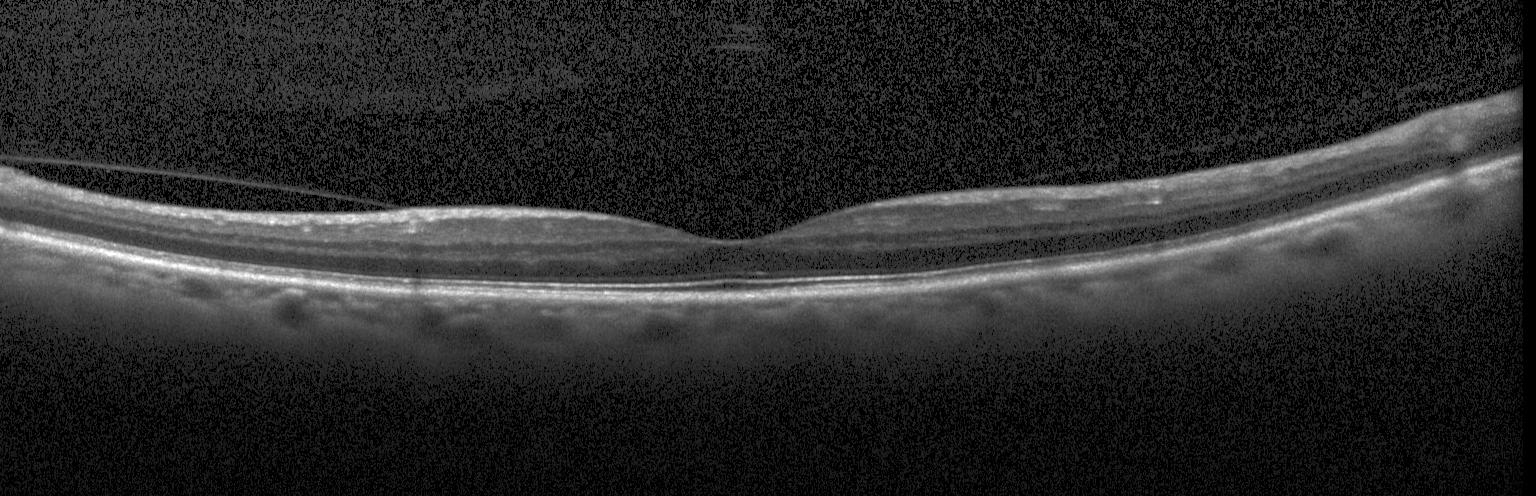 Macular OCT: neither CNV, DME, nor drusen.